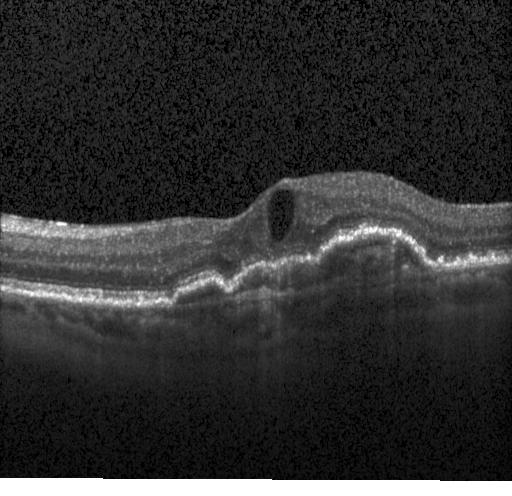 Retinal OCT cross-section showing CNV.